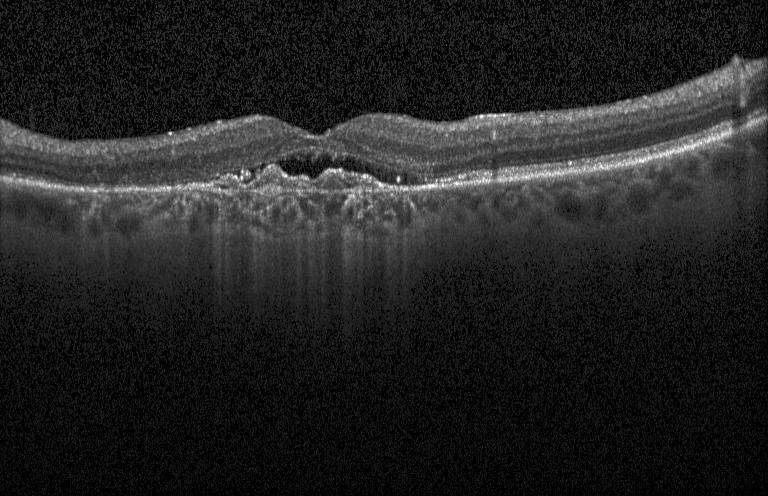
Diagnosis: a choroidal neovascular membrane.